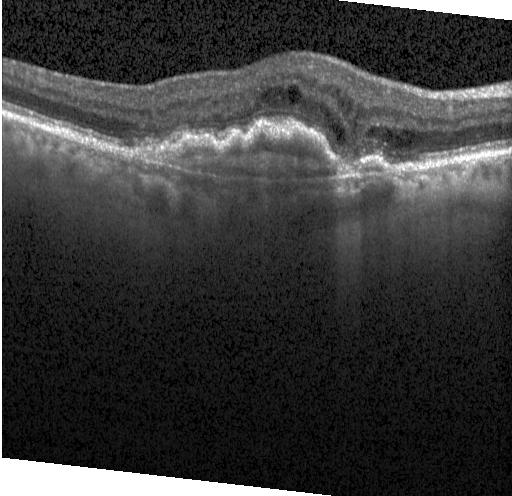 Optical coherence tomography B-scan. Through the macula. Spectral-domain optical coherence tomography. Acquired on a Heidelberg Spectralis.
A choroidal neovascular membrane.